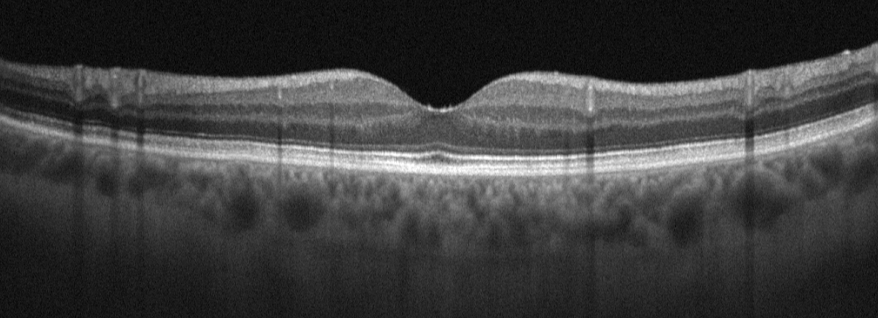
Through the macula · OCT B-scan. OCT finding: absence of AMD, DME, ERM, RAO, RVO, and vitreomacular interface disease.